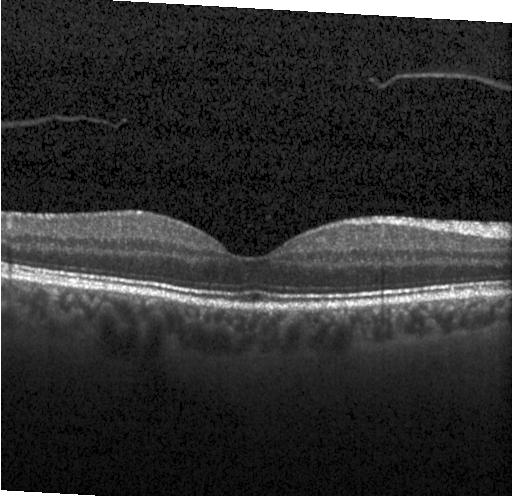 Retinal OCT cross-section; SD-OCT; acquired on a Heidelberg Spectralis; horizontal scan through the fovea.
Diagnosis: no evidence of choroidal neovascularization, diabetic macular edema, or drusen.